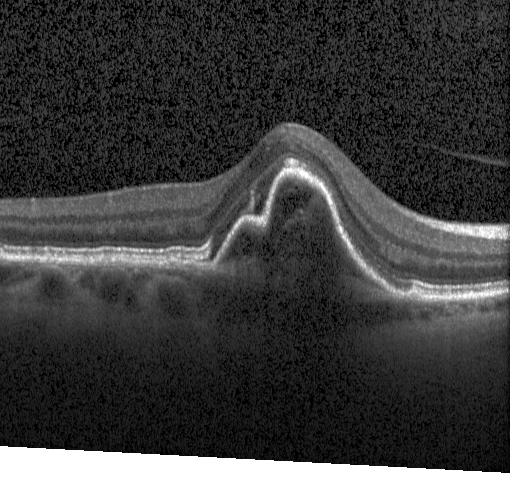 Optical coherence tomography scan. Spectral-domain OCT. Through the macula. Heidelberg Spectralis OCT system — Macular OCT: choroidal neovascularization.